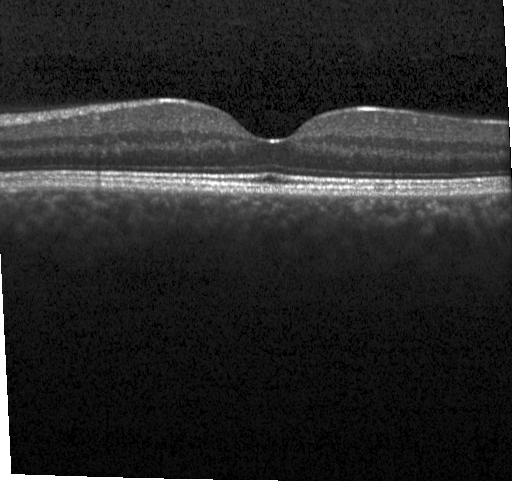
Retinal OCT B-scan. Spectral-domain OCT — The scan shows no choroidal neovascularization, no diabetic macular edema, and no drusen.